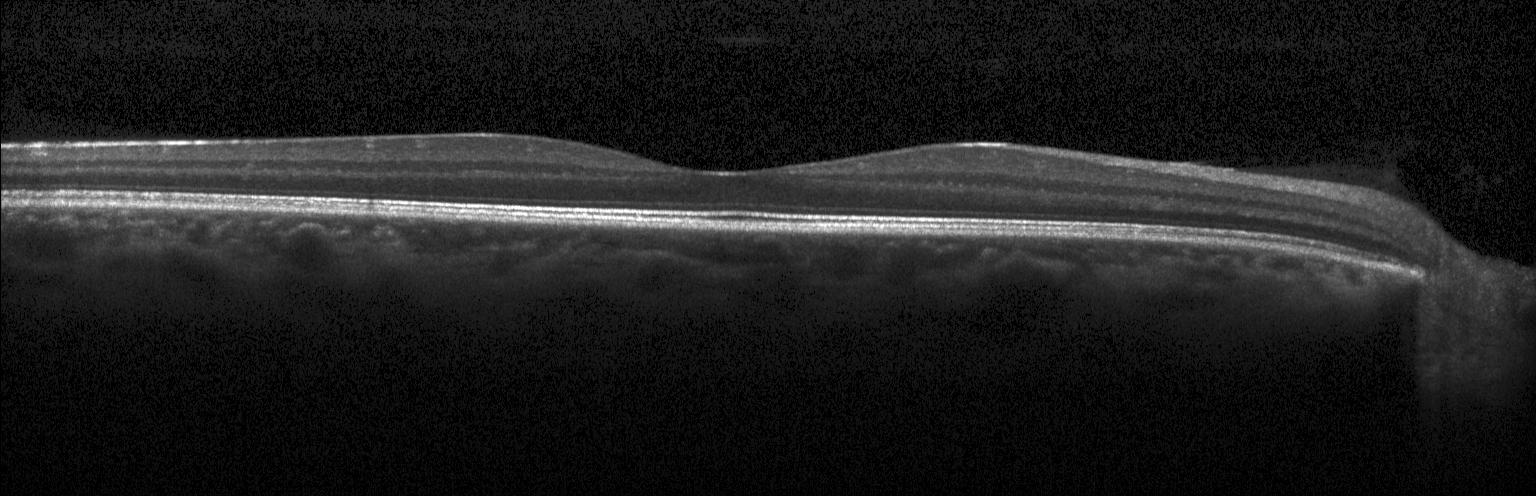 Centered on the fovea; SD-OCT; Heidelberg Spectralis; OCT B-scan — OCT finding: no CNV, DME, or drusen.